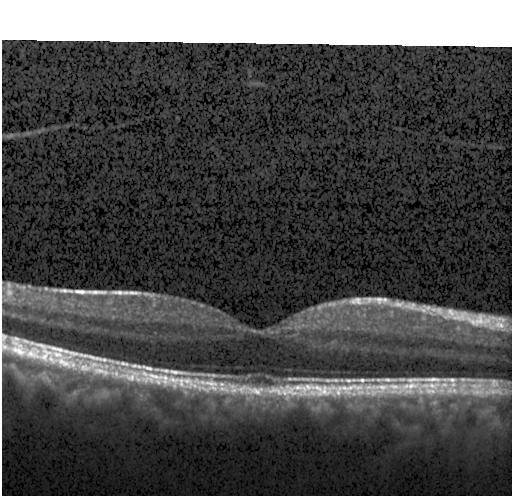 OCT scan showing no evidence of CNV, DME, or drusen.